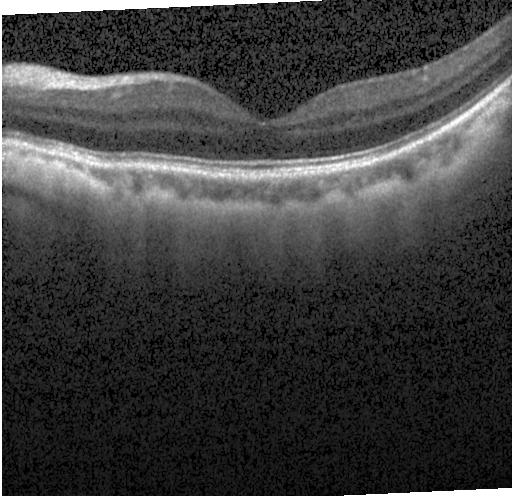
Spectral-domain optical coherence tomography · through the macula · OCT B-scan · instrument: Heidelberg Spectralis — Assessment: no choroidal neovascularization, diabetic macular edema, or drusen.